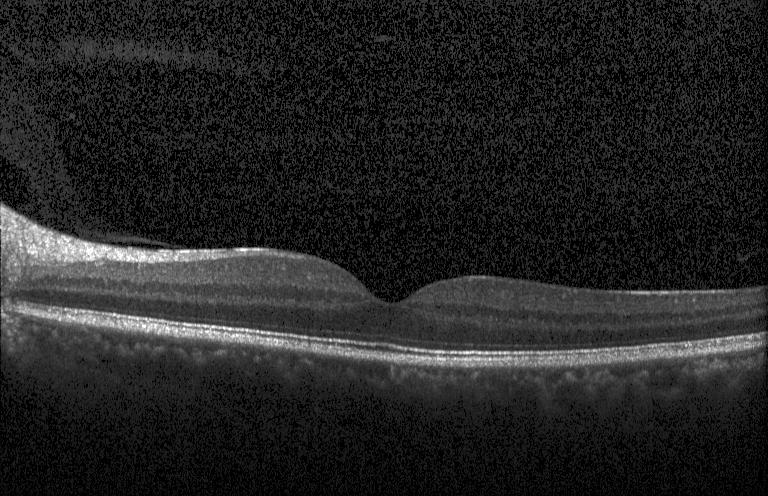

SD-OCT. Retinal OCT cross-section. Through the macula — Finding: no choroidal neovascularization, diabetic macular edema, or drusen.